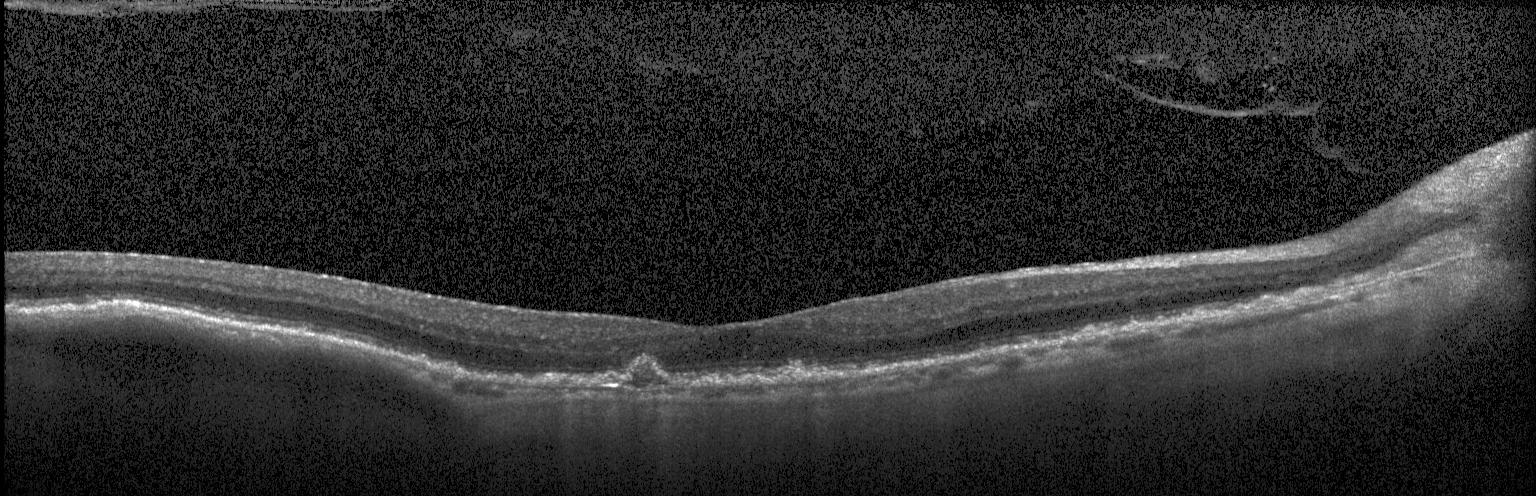 Spectral-domain OCT, acquired on a Heidelberg Spectralis, OCT B-scan
Dx: CNV.